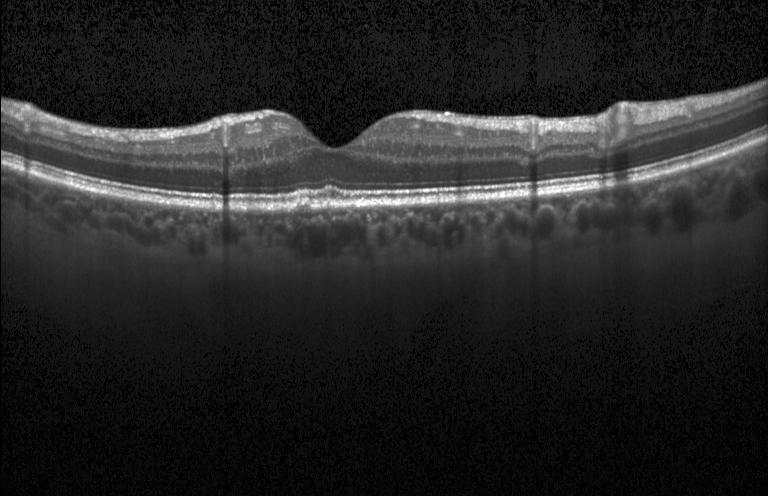 Assessment: multiple drusen.